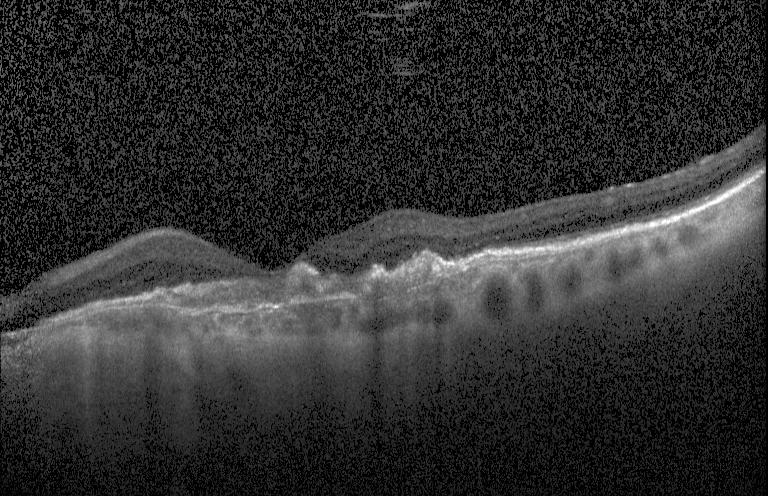

OCT B-scan.
Dx: a choroidal neovascular membrane.